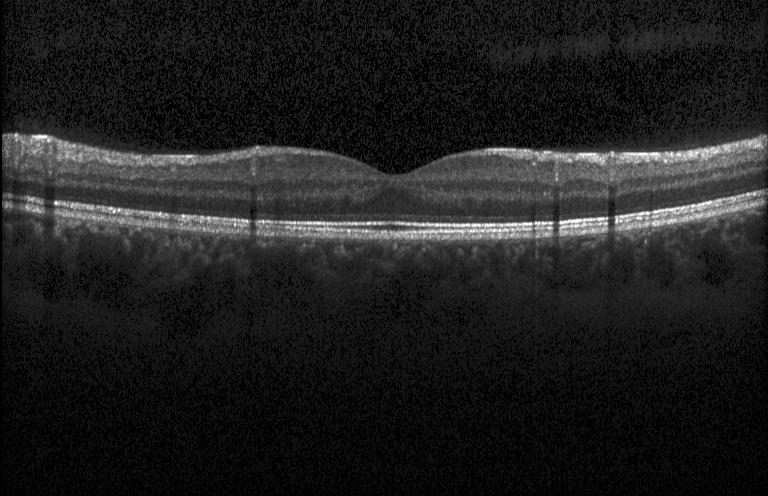 OCT B-scan; macular scan; Heidelberg Spectralis OCT system.
Finding: neither choroidal neovascularization, diabetic macular edema, nor drusen.